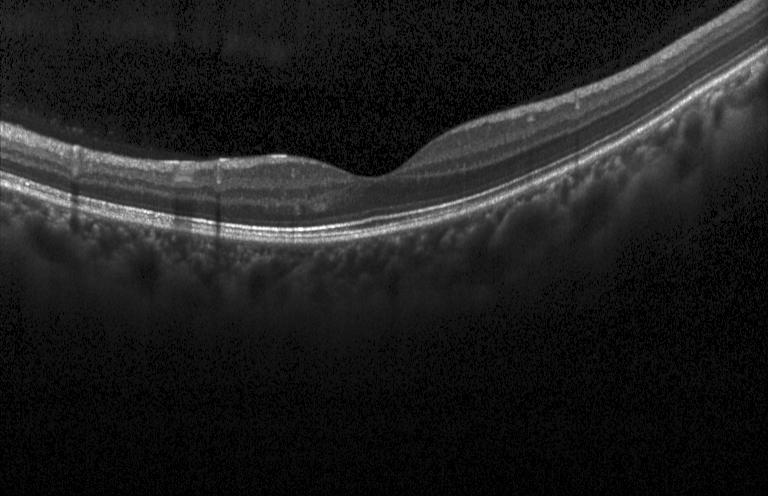

Macular OCT: no CNV, no DME, and no drusen.